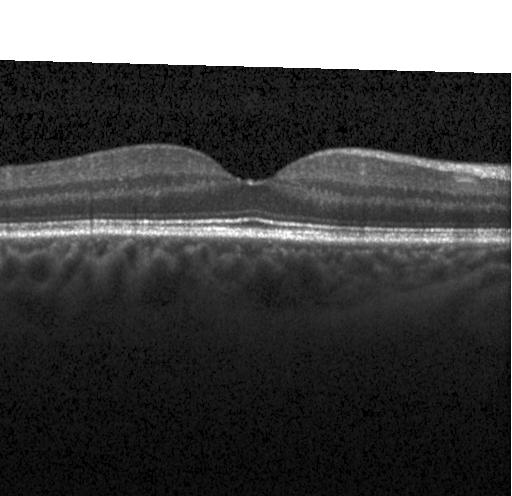
Heidelberg Spectralis; OCT line scan; SD-OCT.
Finding: no evidence of choroidal neovascularization, diabetic macular edema, or drusen.